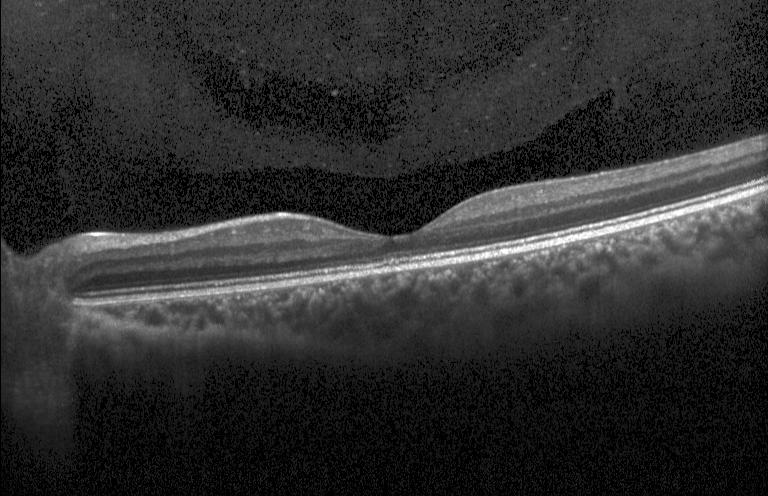

Spectral-domain OCT · instrument: Heidelberg Spectralis · retinal OCT B-scan · centered on the fovea — Finding: no choroidal neovascularization, diabetic macular edema, or drusen.